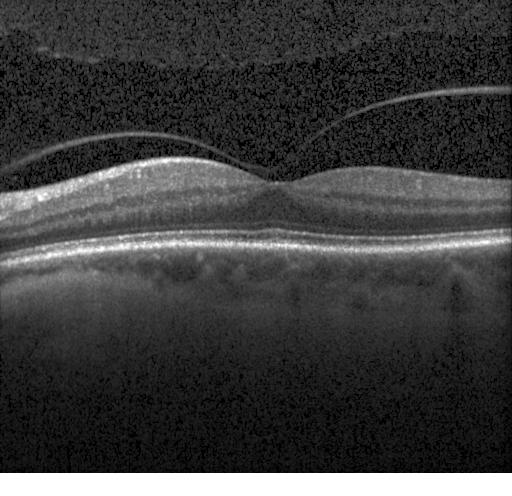

OCT line scan.
This B-scan demonstrates no choroidal neovascularization, diabetic macular edema, or drusen.